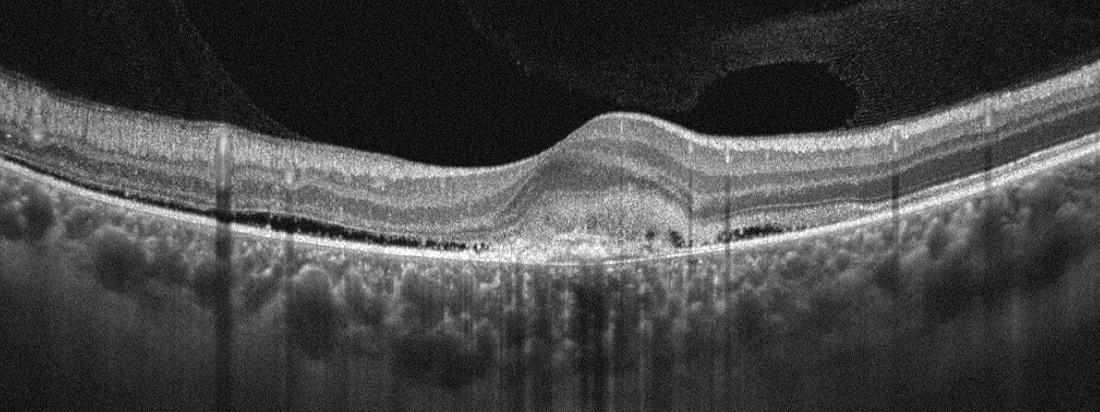
OCT finding: age-related macular degeneration (AMD).